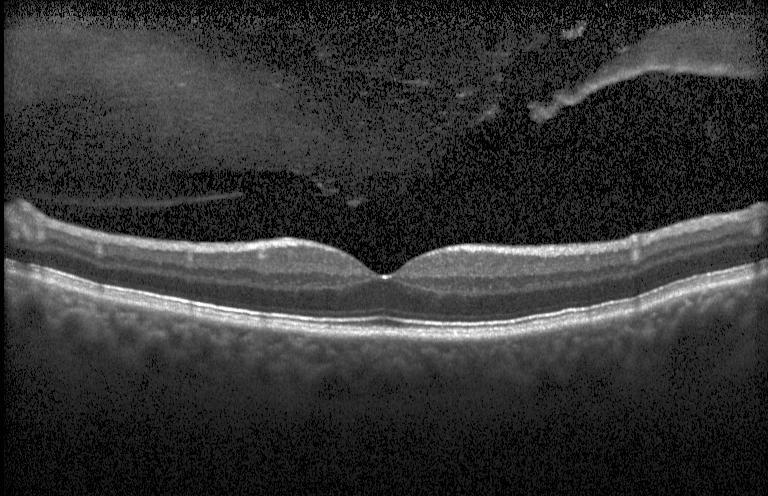 Diagnosis: neither CNV, DME, nor drusen.